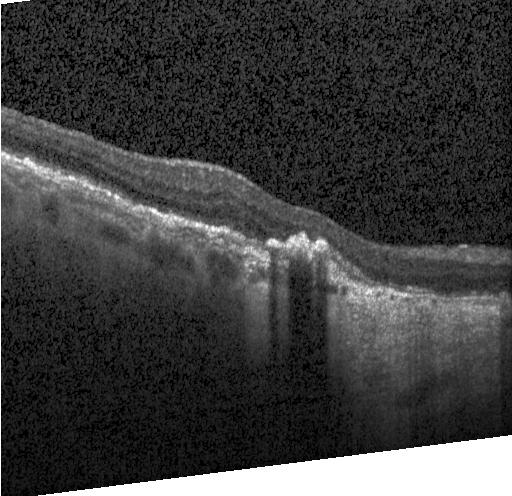
OCT line scan; horizontal scan through the fovea; Heidelberg Spectralis OCT system.
Finding: choroidal neovascularization (CNV).